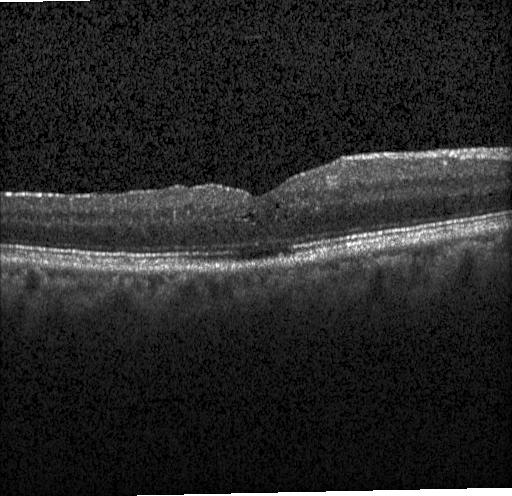

Assessment: diabetic macular edema (DME).